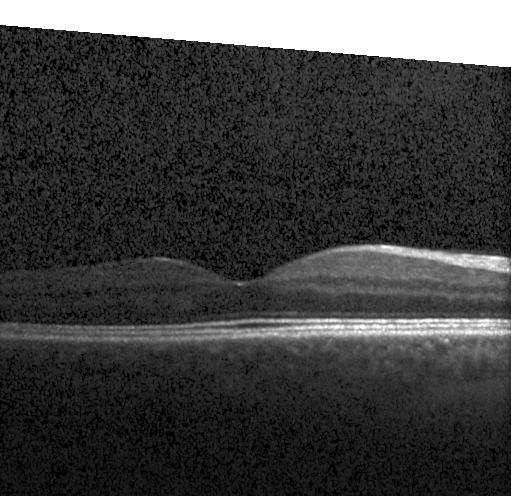

Dx: no evidence of choroidal neovascularization, diabetic macular edema, or drusen.